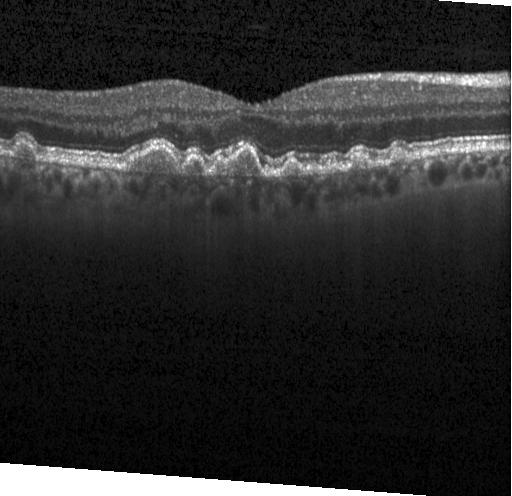

Fovea-centered, spectral-domain OCT, retinal OCT cross-section — The scan shows multiple drusen.